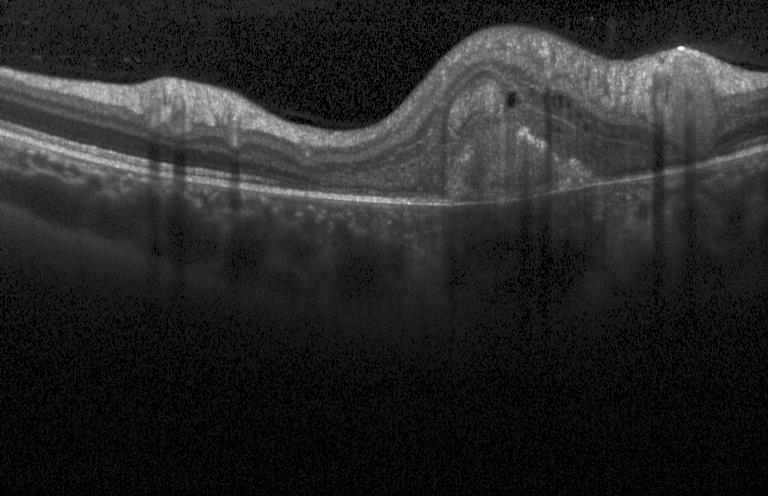

Instrument: Heidelberg Spectralis; optical coherence tomography scan; spectral-domain optical coherence tomography; horizontal scan through the fovea
Impression: CNV.